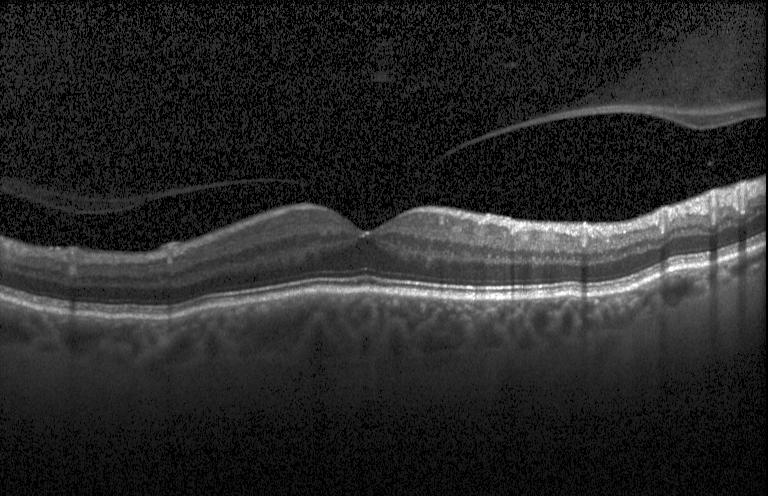 Through the macula · retinal OCT cross-section · instrument: Heidelberg Spectralis · spectral-domain optical coherence tomography.
The scan shows no choroidal neovascularization, diabetic macular edema, or drusen.